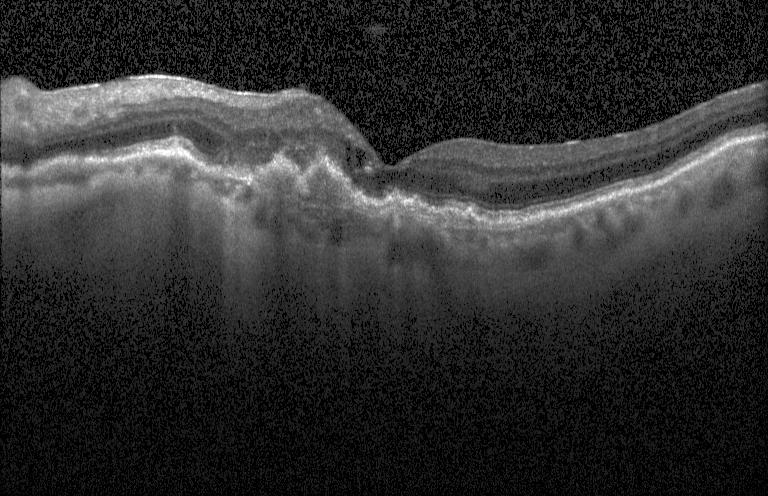
Retinal OCT B-scan. Spectral-domain optical coherence tomography. Heidelberg Spectralis.
A choroidal neovascular membrane.